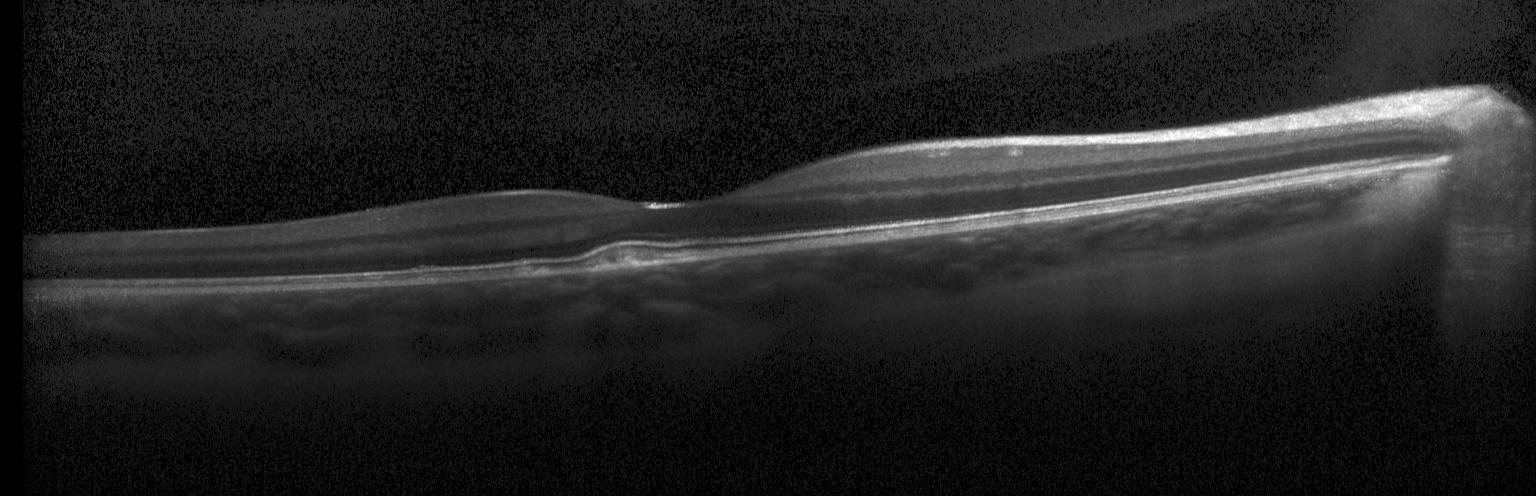

Finding: sub-RPE drusenoid deposits.